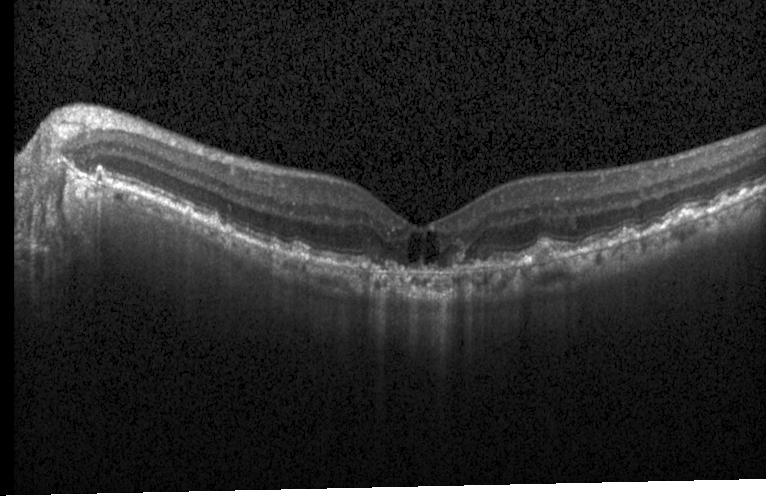 Optical coherence tomography B-scan
Impression: CNV.